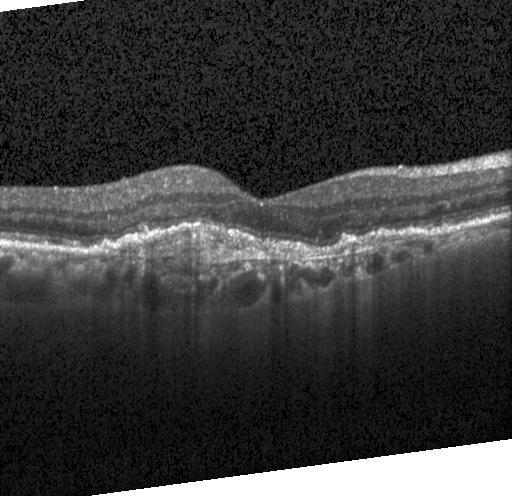

Acquired on a Heidelberg Spectralis · optical coherence tomography scan.
This B-scan demonstrates choroidal neovascularization.